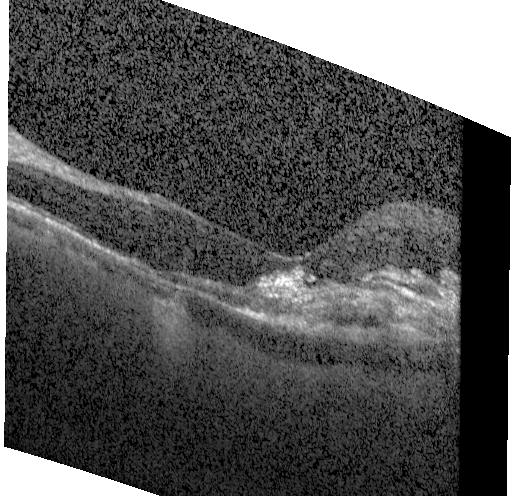

OCT B-scan — Dx: a choroidal neovascular membrane.